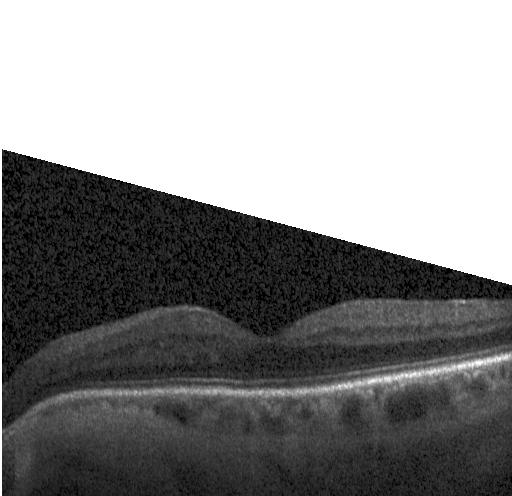 Spectral-domain OCT, Heidelberg Spectralis OCT system, retinal OCT cross-section, macular scan — Impression: no CNV, no DME, and no drusen.